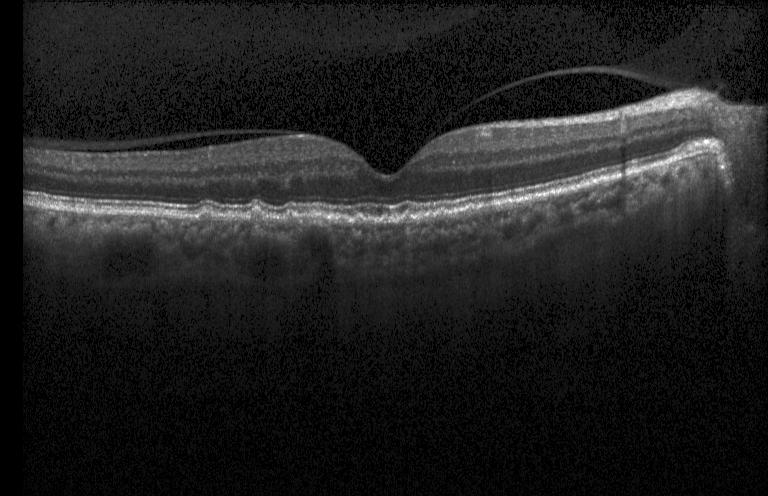

OCT B-scan — Diagnosis: sub-RPE drusenoid deposits.